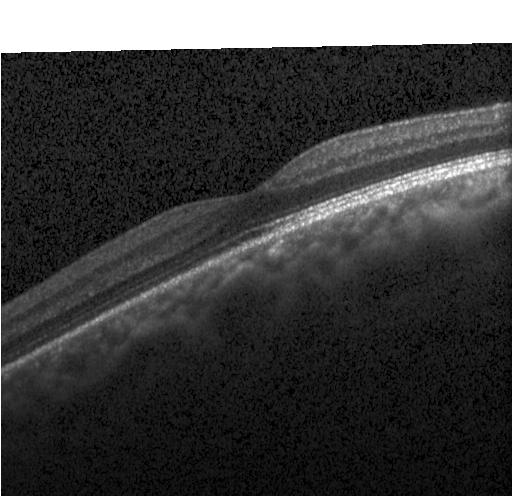
Optical coherence tomography scan
Finding: no evidence of CNV, DME, or drusen.